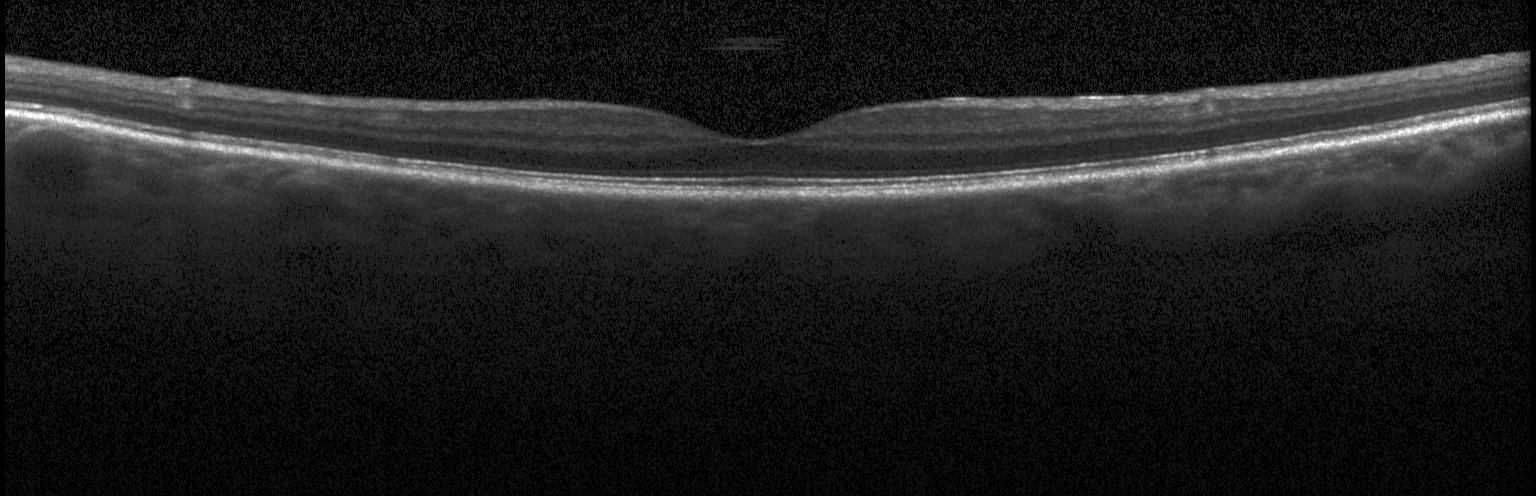
SD-OCT. OCT B-scan. Acquired on a Heidelberg Spectralis.
Impression: no evidence of choroidal neovascularization, diabetic macular edema, or drusen.